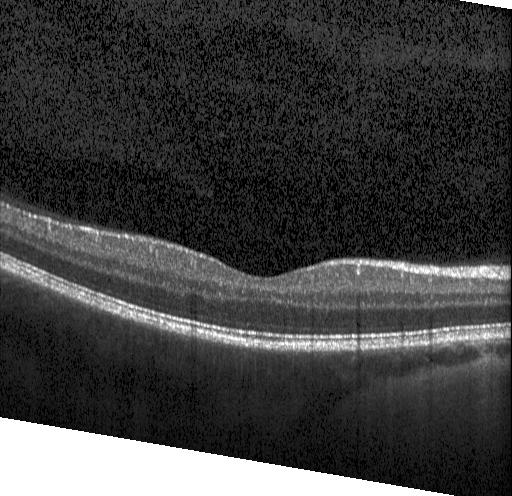

OCT line scan. Spectral-domain optical coherence tomography.
OCT finding: no choroidal neovascularization, diabetic macular edema, or drusen.